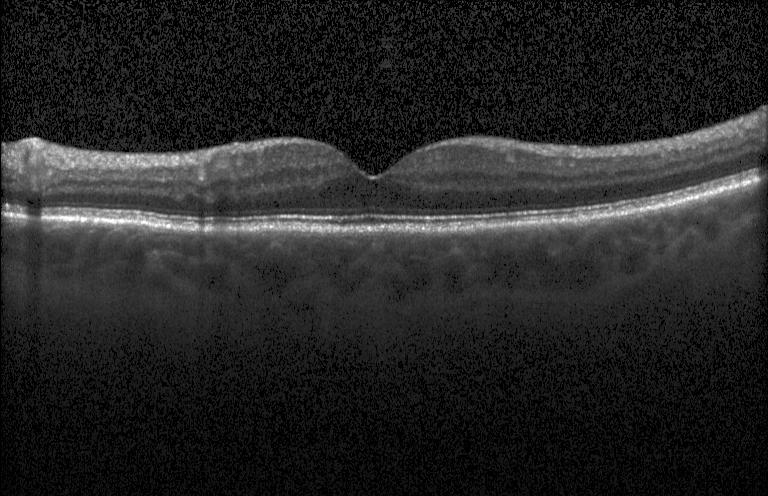 Diagnosis: neither choroidal neovascularization, diabetic macular edema, nor drusen.